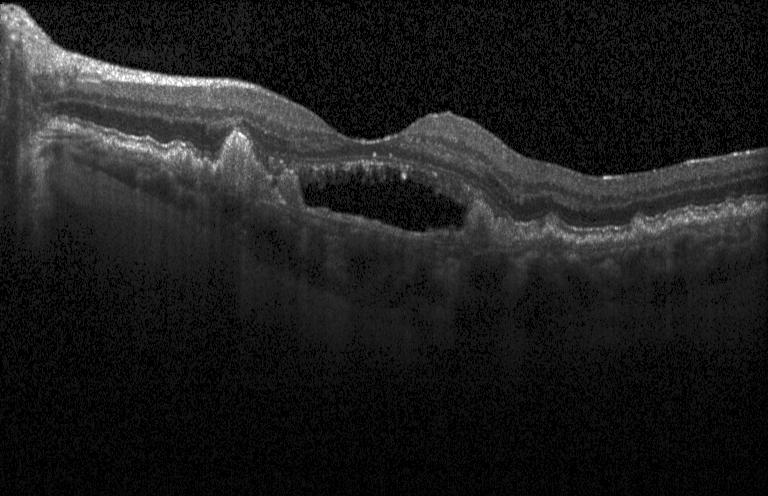

Through the macula; retinal OCT B-scan; instrument: Heidelberg Spectralis
Finding: choroidal neovascularization.